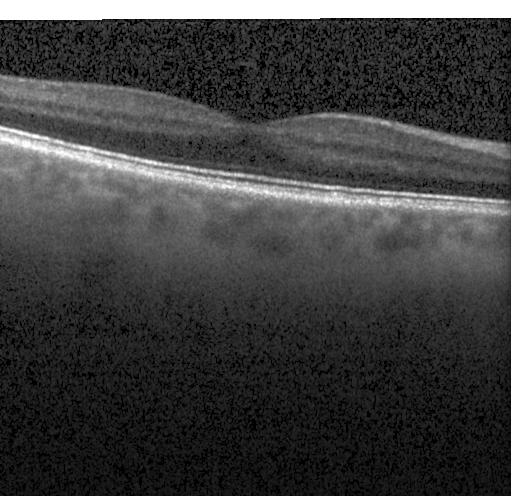
Spectral-domain OCT, Heidelberg Spectralis OCT system, OCT B-scan. Dx: neither choroidal neovascularization, diabetic macular edema, nor drusen.